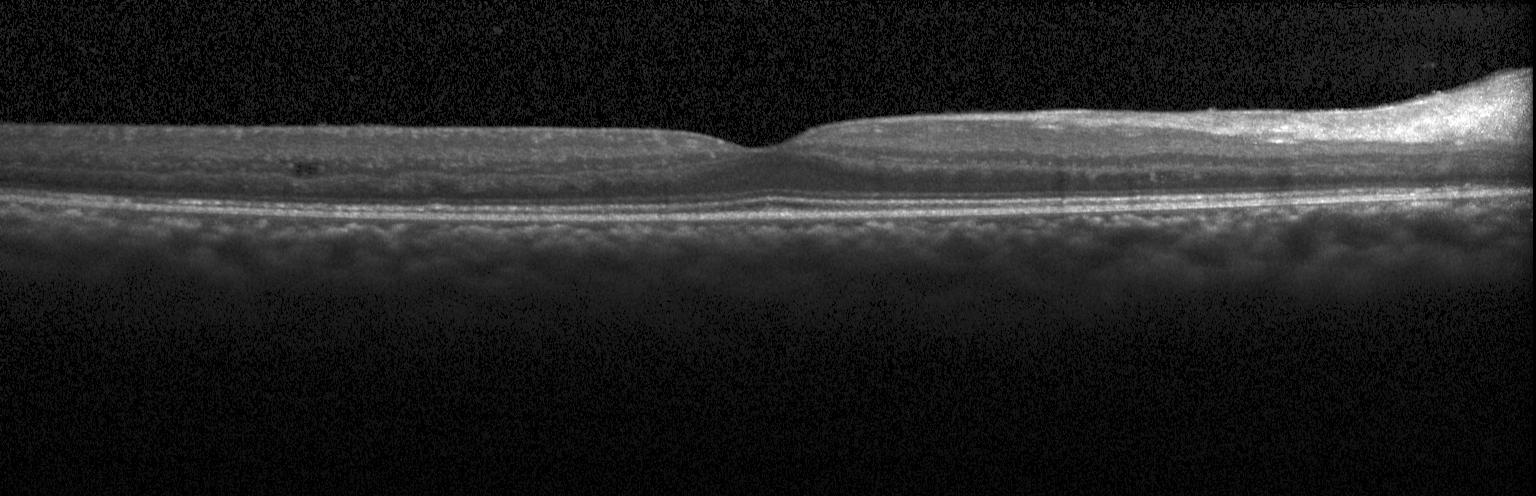 Optical coherence tomography scan, spectral-domain optical coherence tomography.
Diagnosis: DME.